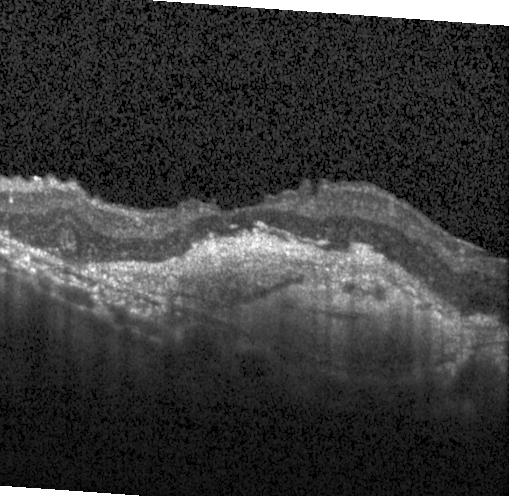 Through the macula · optical coherence tomography scan · instrument: Heidelberg Spectralis · spectral-domain optical coherence tomography
Impression: a choroidal neovascular membrane.